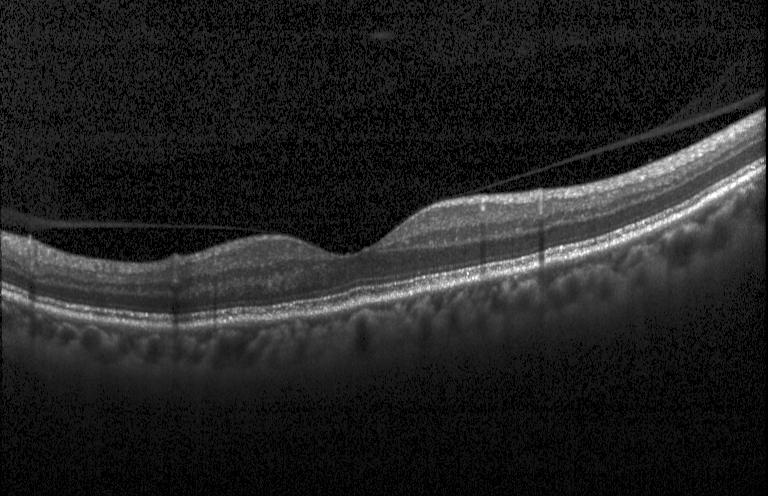
Diagnosis: neither choroidal neovascularization, diabetic macular edema, nor drusen.